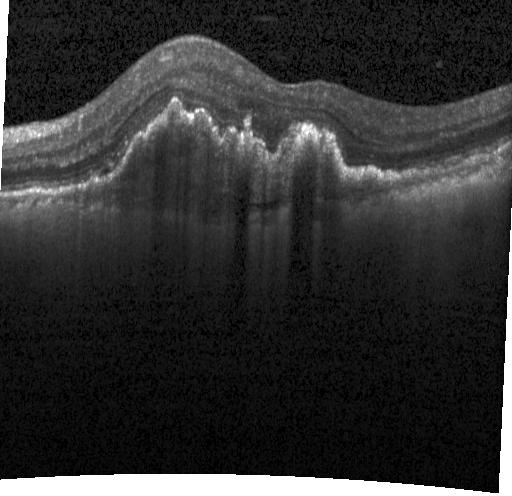

Spectral-domain OCT B-scan: a choroidal neovascular membrane.